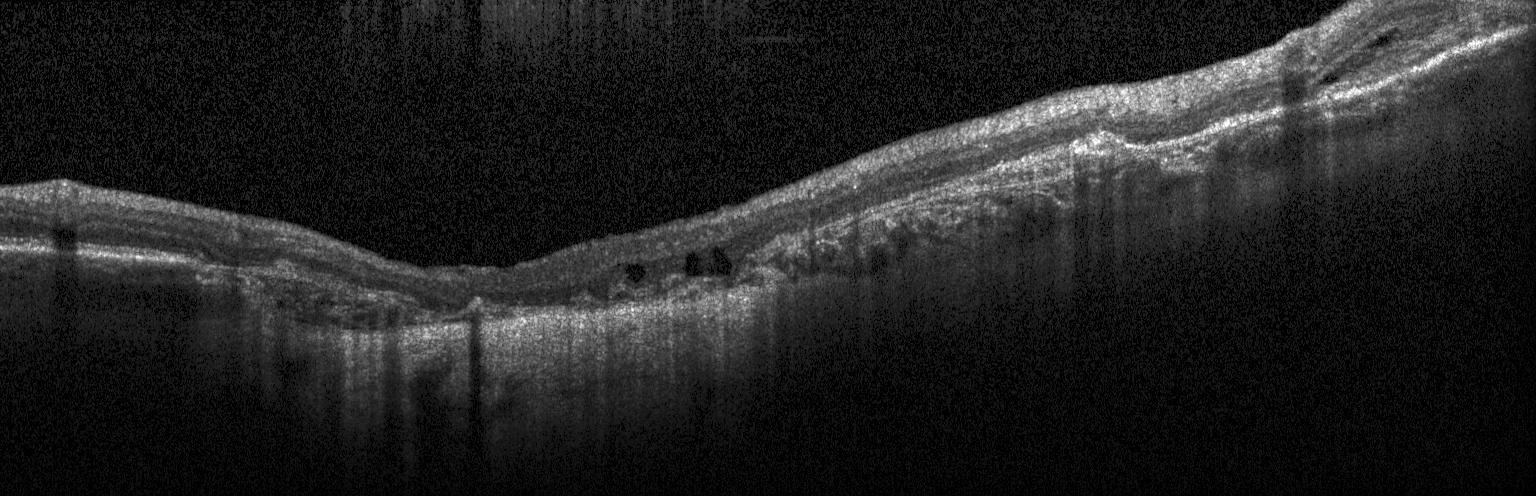

Heidelberg Spectralis OCT system; OCT line scan; fovea-centered; spectral-domain OCT.
A choroidal neovascular membrane.